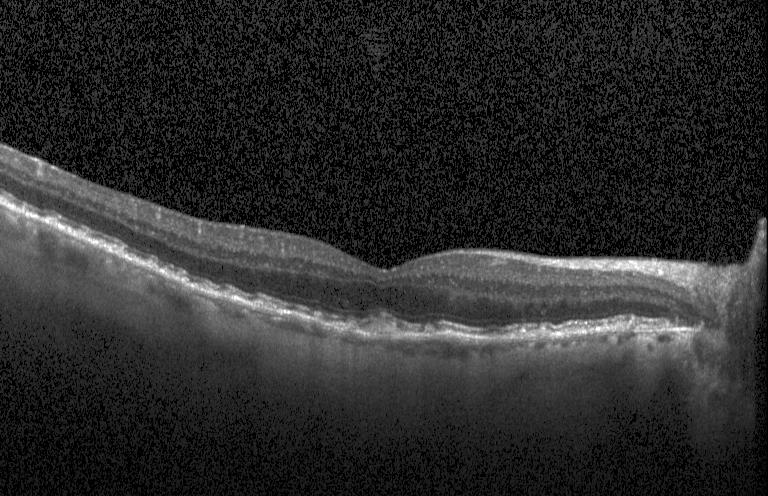 The scan shows drusen.